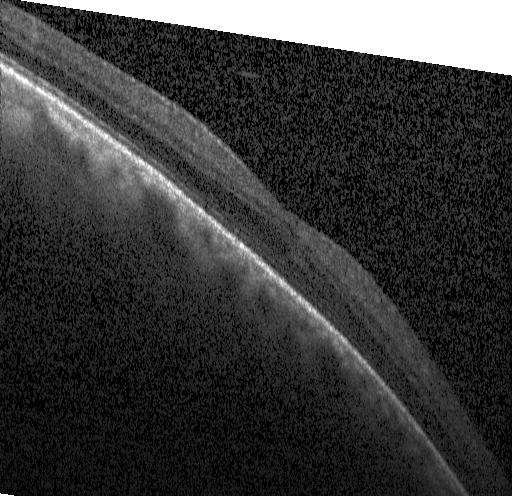

Retinal OCT cross-section.
This B-scan demonstrates no evidence of choroidal neovascularization, diabetic macular edema, or drusen.